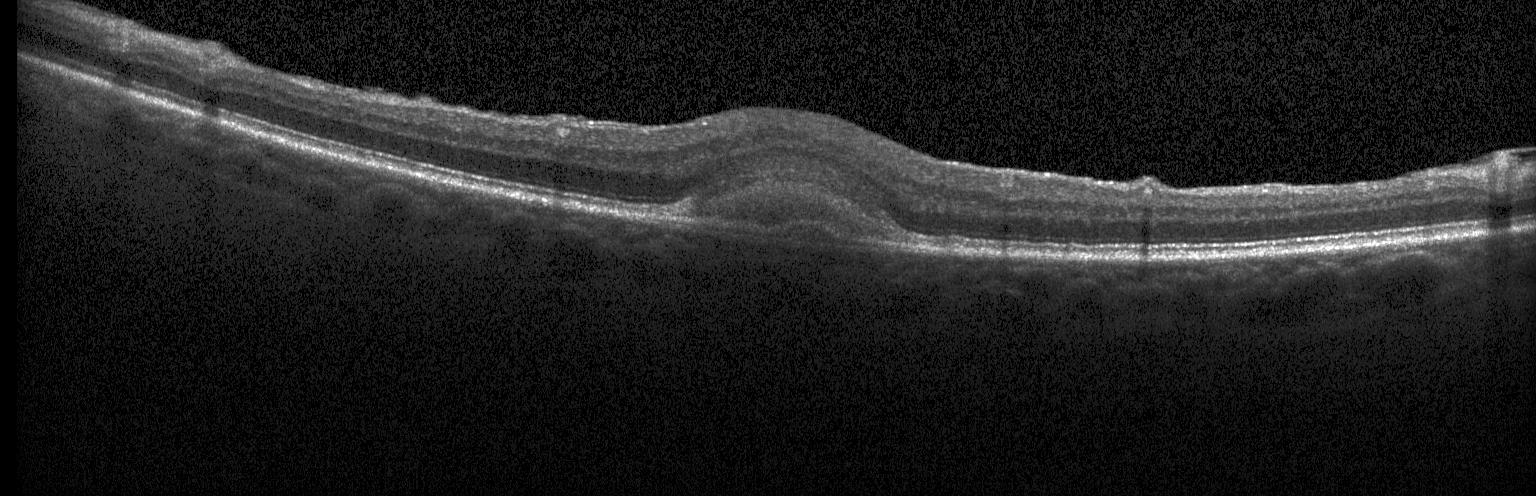

Heidelberg Spectralis OCT system; retinal OCT cross-section — Finding: CNV.